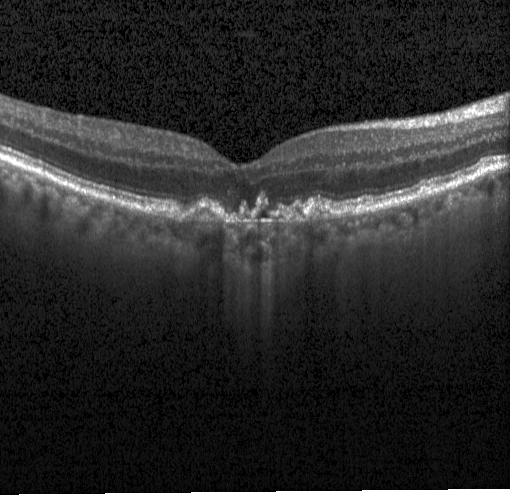
Instrument: Heidelberg Spectralis. Retinal OCT B-scan. Centered on the fovea — Assessment: choroidal neovascularization.